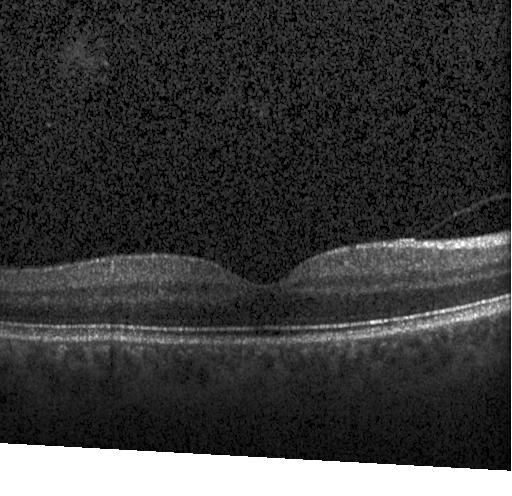
Retinal OCT cross-section showing no evidence of choroidal neovascularization, diabetic macular edema, or drusen.